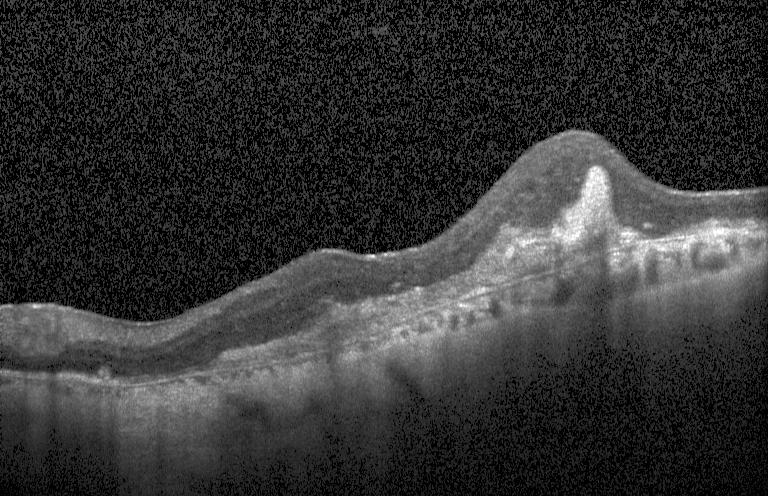 OCT B-scan, SD-OCT, instrument: Heidelberg Spectralis. Impression: a choroidal neovascular membrane.